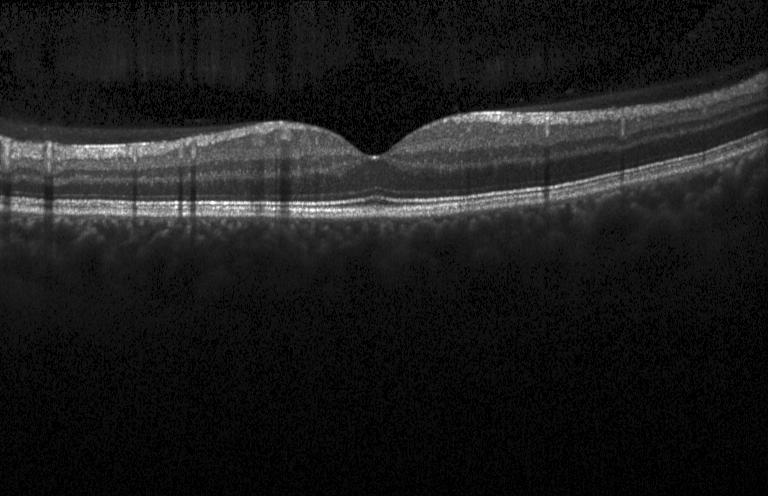
Impression: no choroidal neovascularization, diabetic macular edema, or drusen.